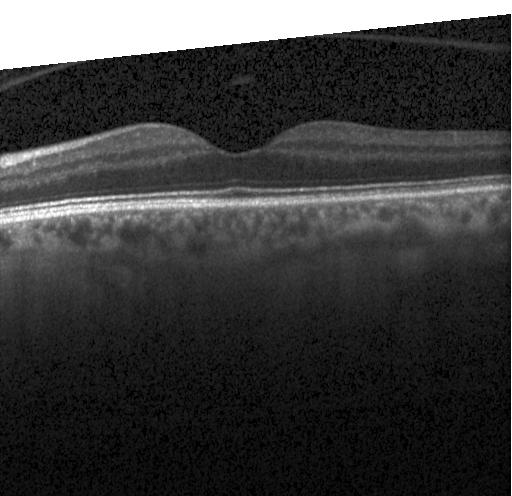 OCT finding: no choroidal neovascularization, no diabetic macular edema, and no drusen.